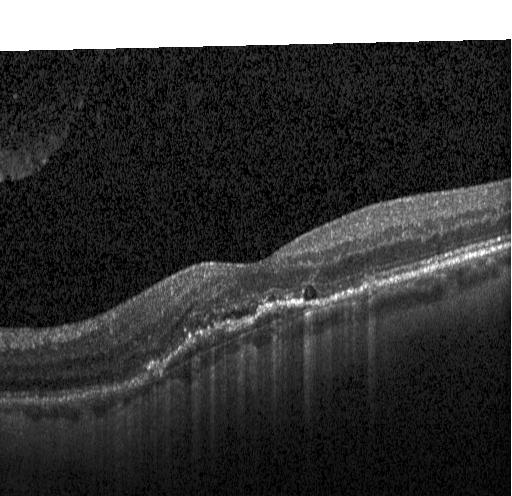
Instrument: Heidelberg Spectralis · OCT line scan · spectral-domain OCT. Finding: choroidal neovascularization (CNV).